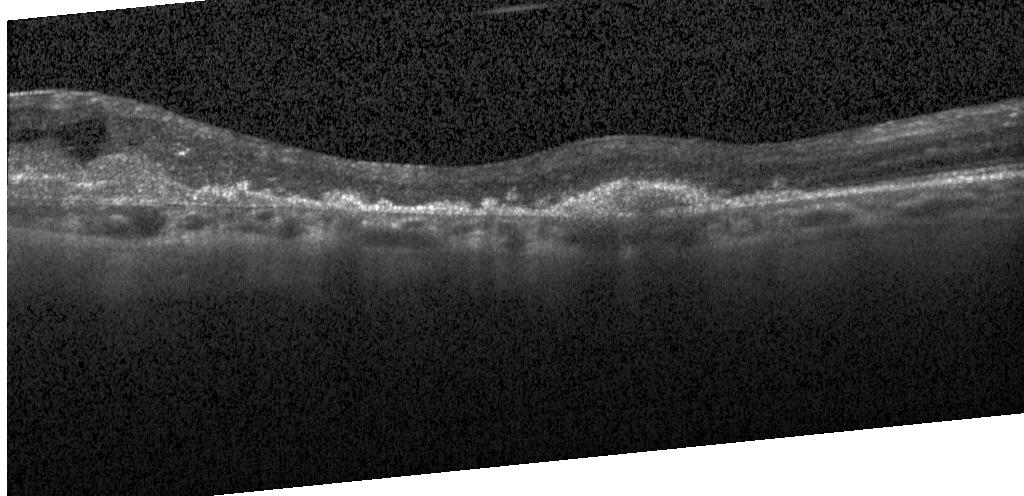
Spectral-domain OCT B-scan: a choroidal neovascular membrane.